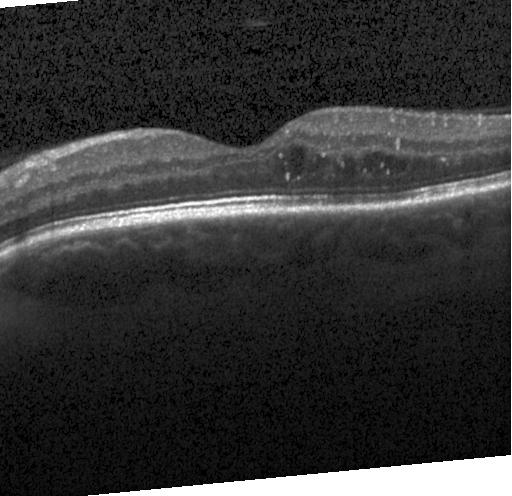 Acquired on a Heidelberg Spectralis. Retinal OCT B-scan
Dx: DME.